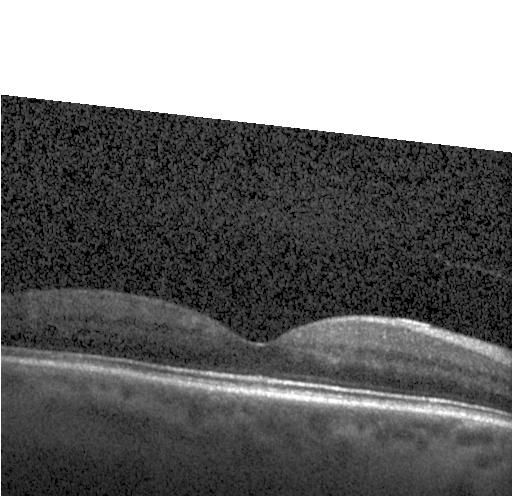
Optical coherence tomography scan.
Impression: no choroidal neovascularization, diabetic macular edema, or drusen.